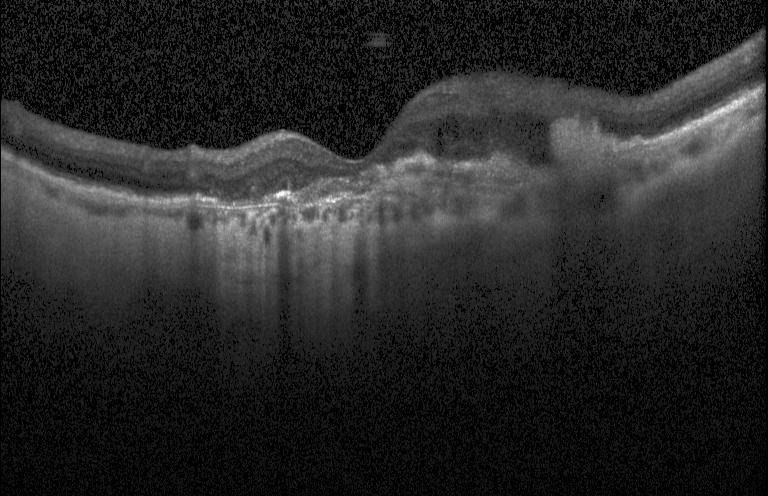 Heidelberg Spectralis OCT system, horizontal scan through the fovea, retinal OCT B-scan, spectral-domain optical coherence tomography.
Finding: a choroidal neovascular membrane.